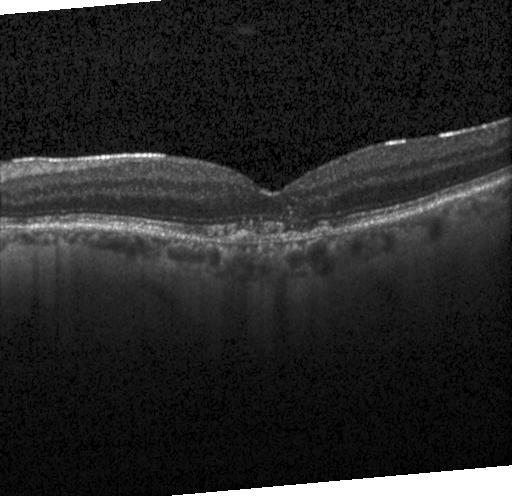 Spectral-domain OCT B-scan: choroidal neovascularization (CNV).